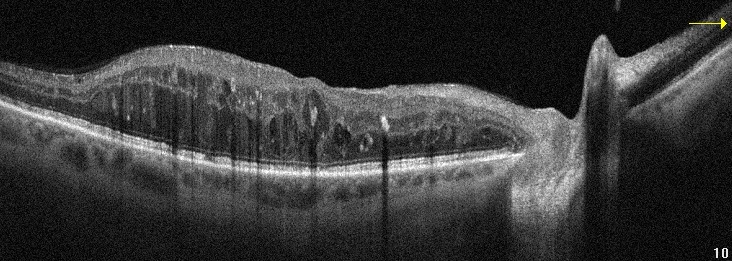

Retinal OCT cross-section. Through the macula. Optovue Avanti RTVue XR — Diagnosis: DME.